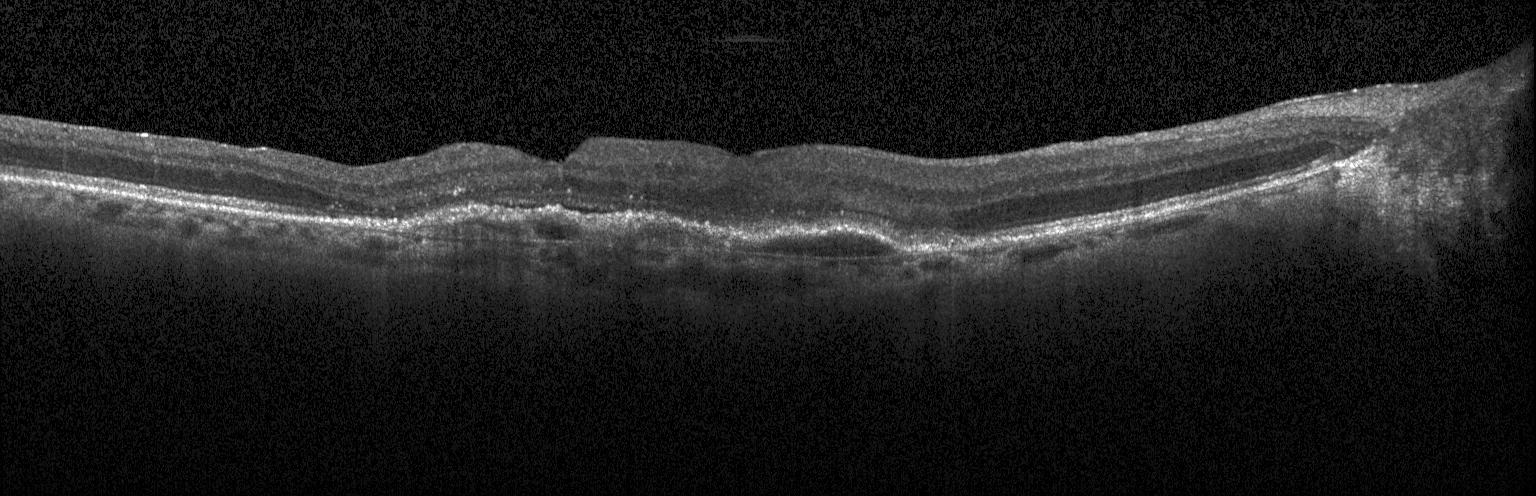
Acquired on a Heidelberg Spectralis · spectral-domain optical coherence tomography · macular scan · optical coherence tomography B-scan
Assessment: a choroidal neovascular membrane.